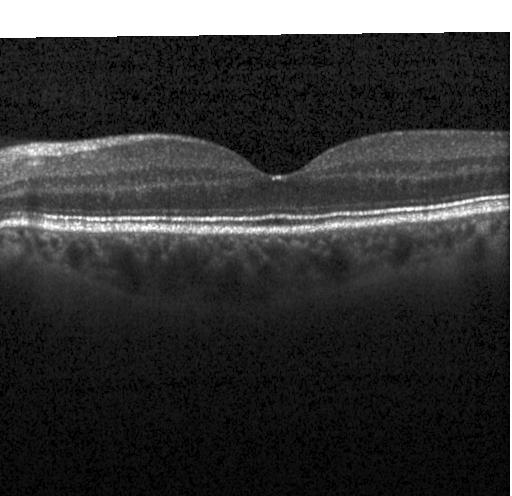 OCT line scan · Heidelberg Spectralis OCT system — This B-scan demonstrates no evidence of choroidal neovascularization, diabetic macular edema, or drusen.